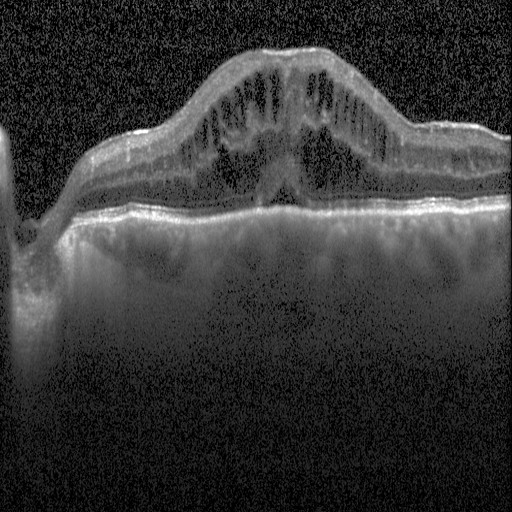 Retinal OCT B-scan. Finding: diabetic macular edema (DME).